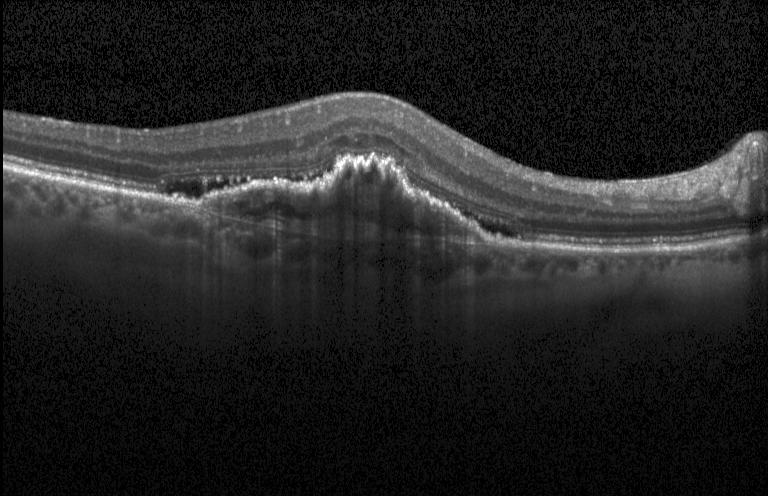 Acquired on a Heidelberg Spectralis · optical coherence tomography B-scan · macular scan
Macular OCT: CNV.